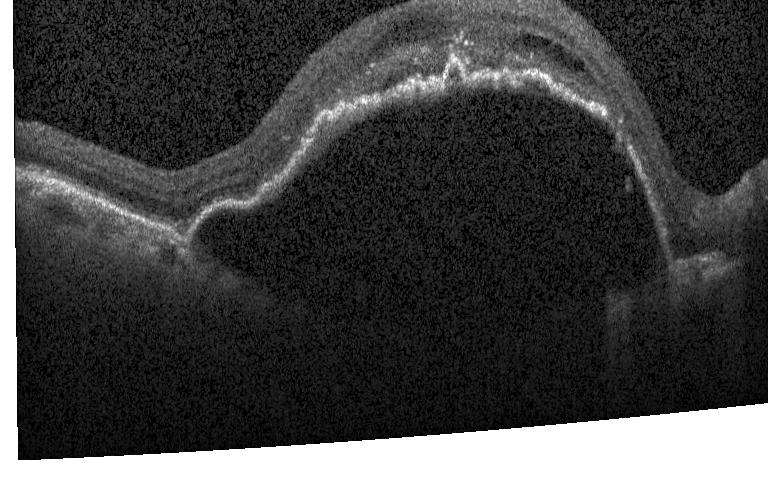 Spectral-domain optical coherence tomography; instrument: Heidelberg Spectralis; horizontal scan through the fovea; OCT B-scan
OCT finding: a choroidal neovascular membrane.